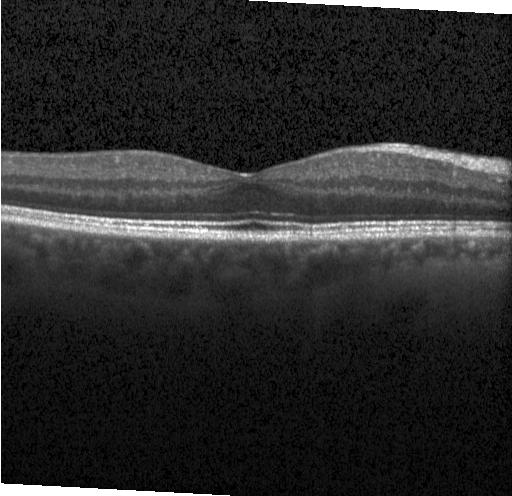
OCT B-scan. Assessment: neither CNV, DME, nor drusen.